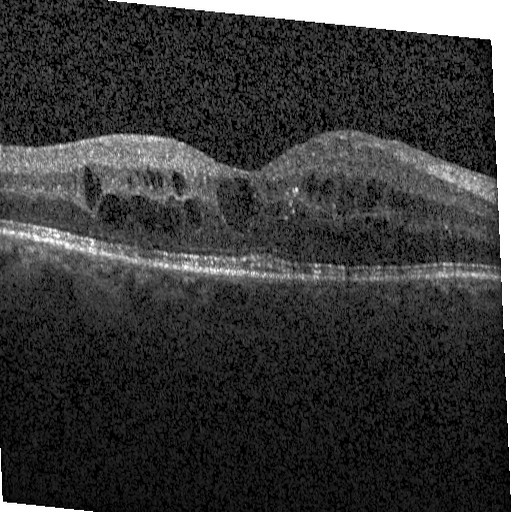

OCT B-scan. Macular scan. Acquired on a Heidelberg Spectralis
Finding: DME.